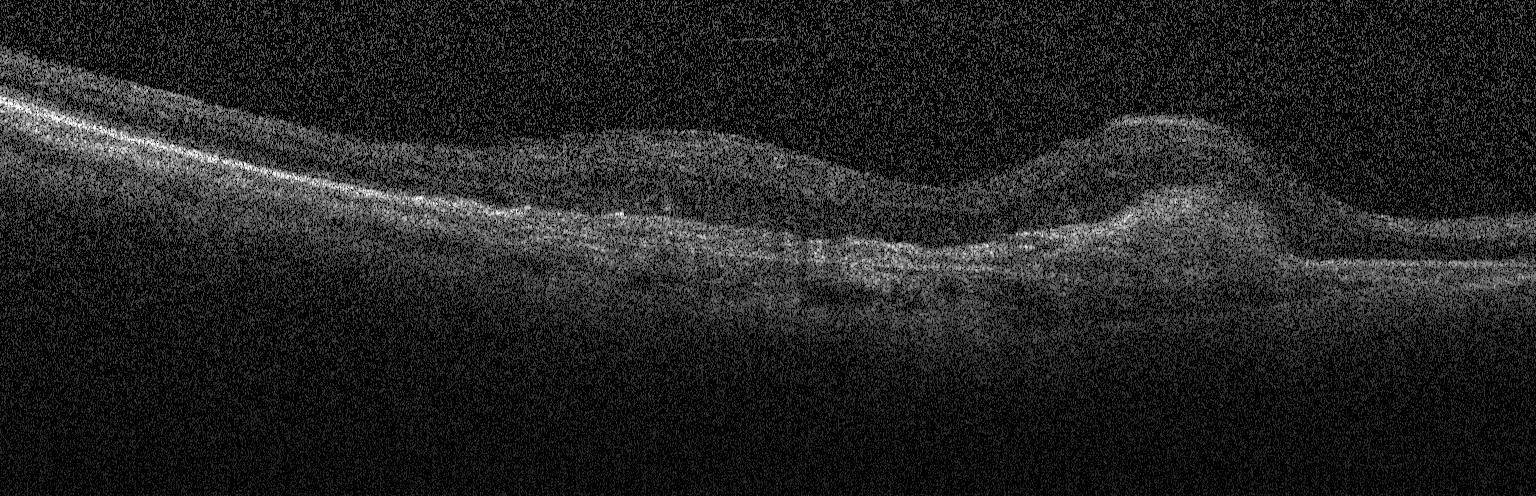
Assessment: choroidal neovascularization.